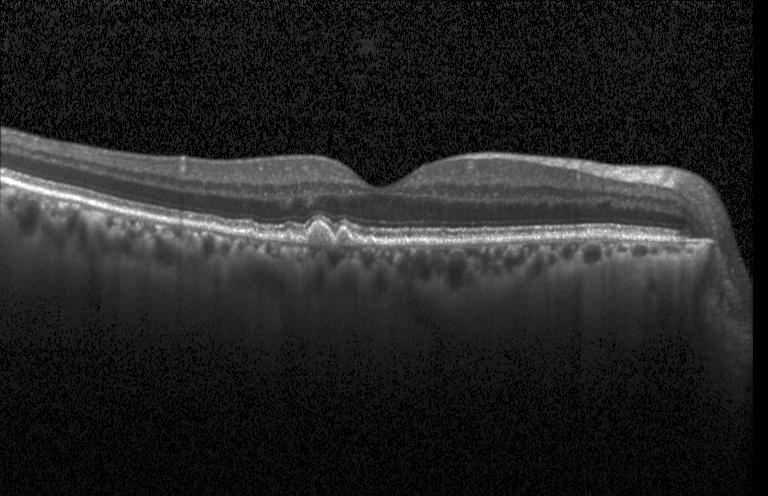

Optical coherence tomography scan. Heidelberg Spectralis OCT system.
Impression: sub-RPE drusenoid deposits.